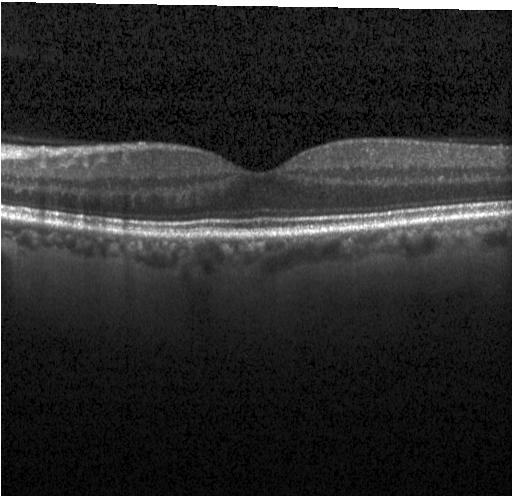 Assessment: no CNV, DME, or drusen.